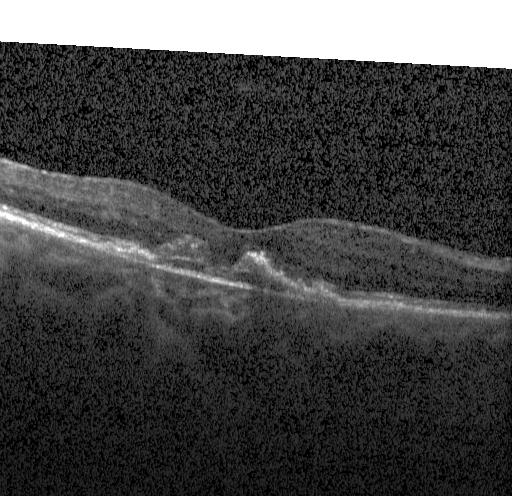

Instrument: Heidelberg Spectralis; optical coherence tomography scan; spectral-domain OCT; centered on the fovea.
A choroidal neovascular membrane.